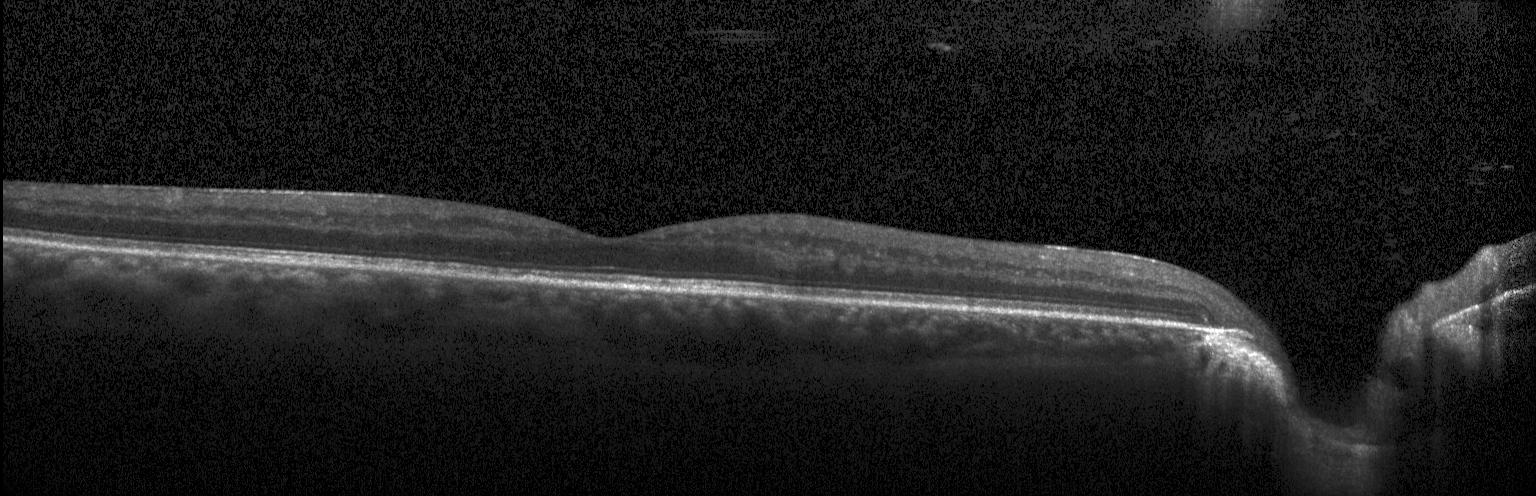
Neither choroidal neovascularization, diabetic macular edema, nor drusen.